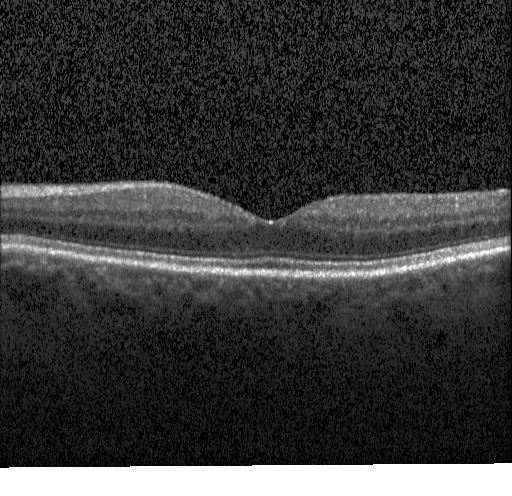

OCT finding: no choroidal neovascularization, diabetic macular edema, or drusen.